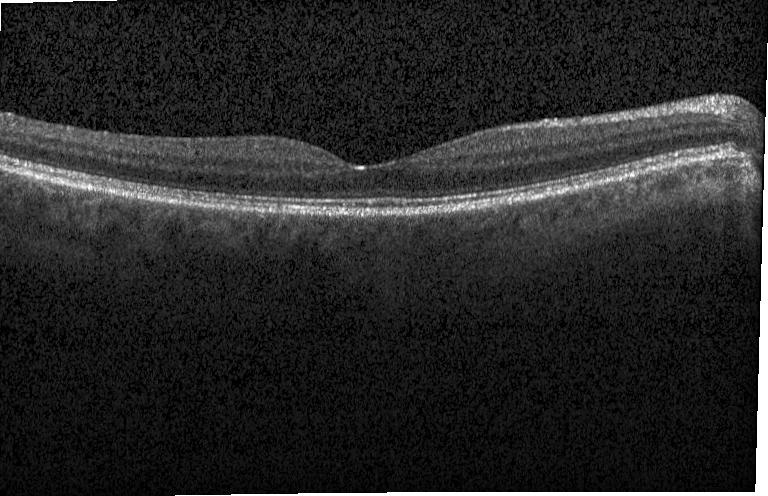

Retinal OCT cross-section. Impression: no choroidal neovascularization, no diabetic macular edema, and no drusen.